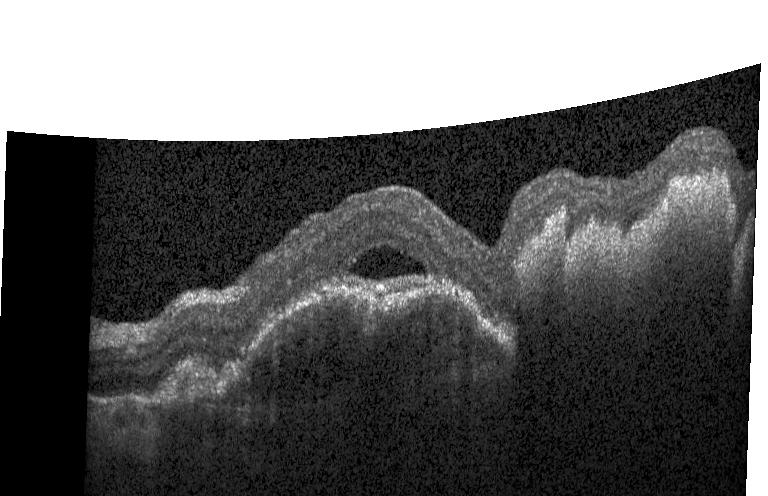

OCT B-scan; acquired on a Heidelberg Spectralis; fovea-centered
Macular OCT: CNV.